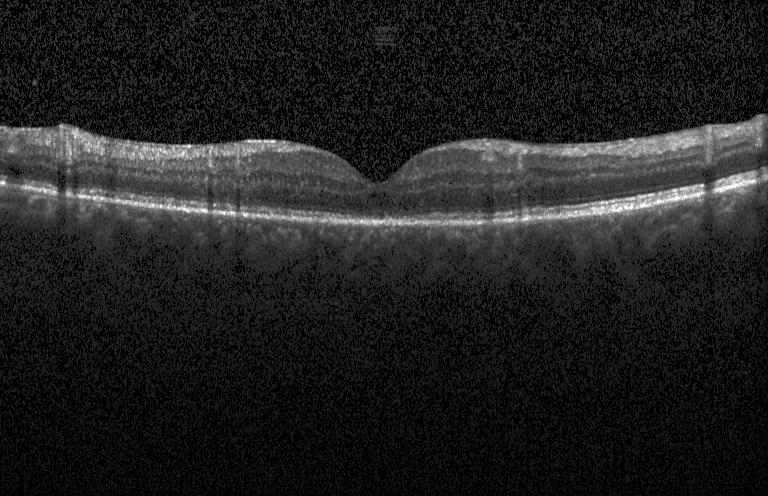 Diagnosis: no choroidal neovascularization, no diabetic macular edema, and no drusen.